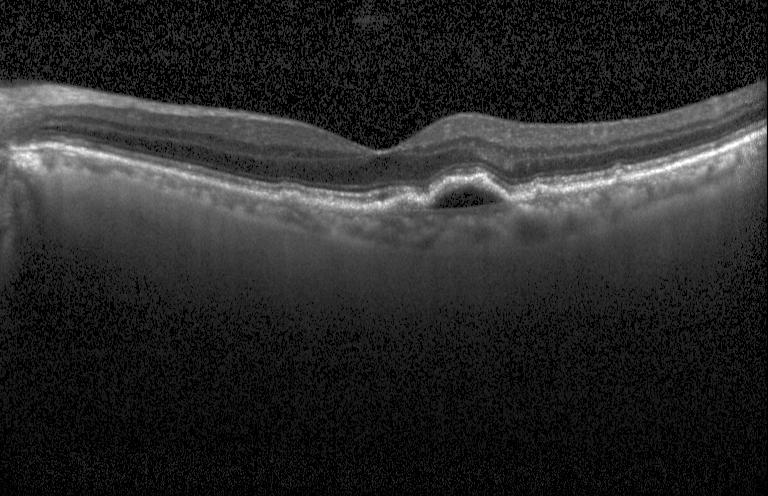 The scan shows a choroidal neovascular membrane.